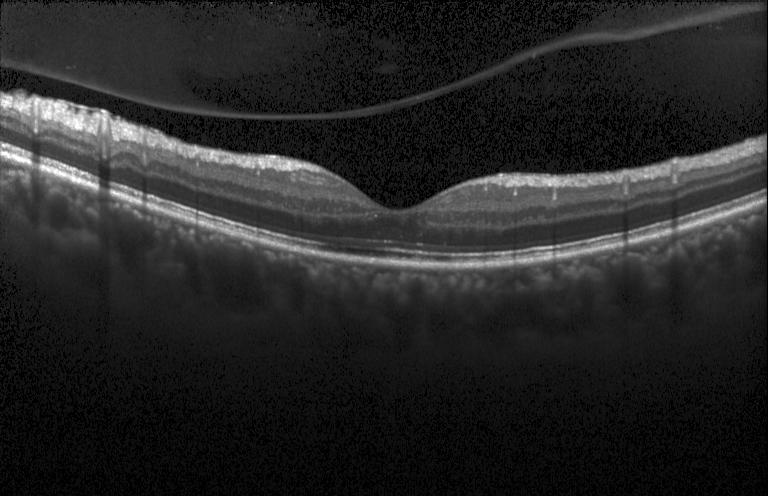

Diagnosis: no evidence of choroidal neovascularization, diabetic macular edema, or drusen.